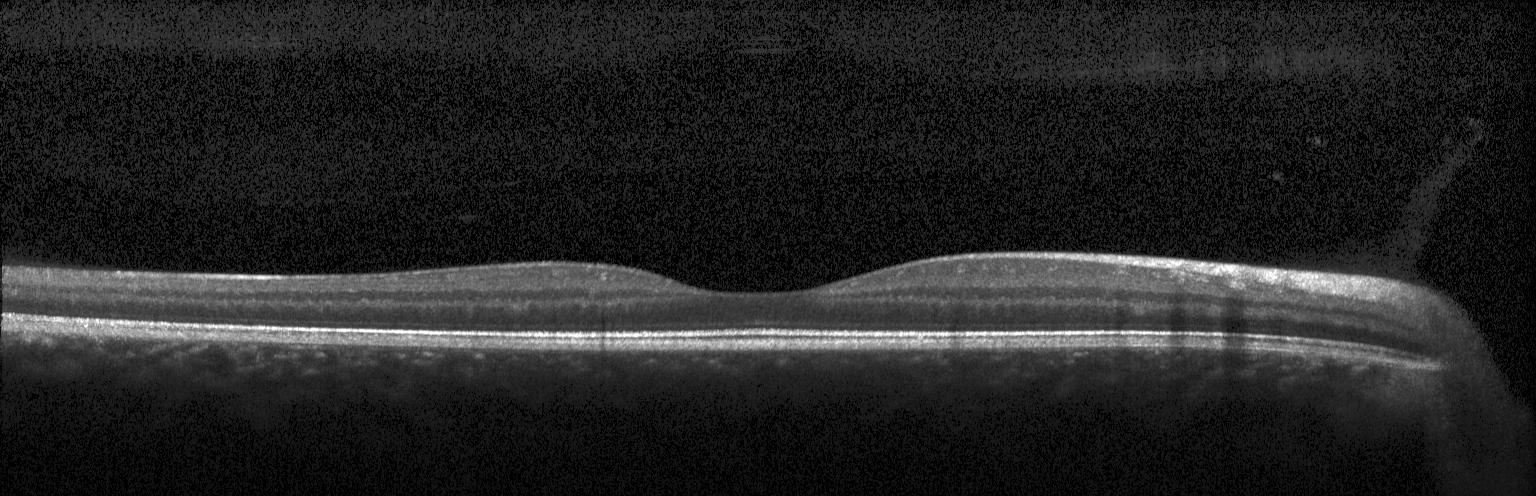 Spectral-domain OCT B-scan: no evidence of choroidal neovascularization, diabetic macular edema, or drusen.